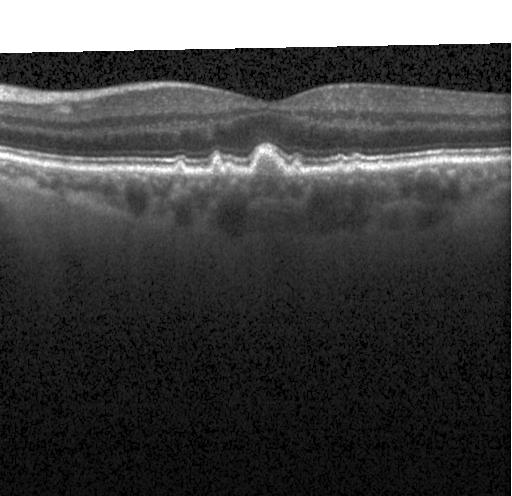

OCT B-scan. Dx: sub-RPE drusenoid deposits.